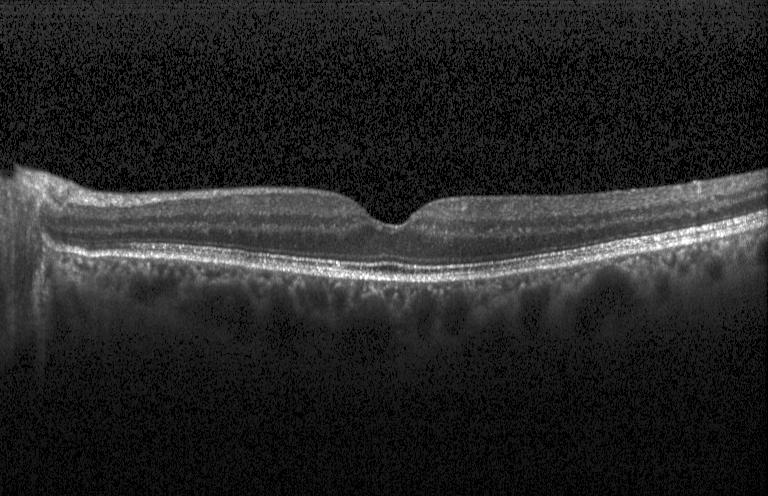 Retinal OCT cross-section showing no choroidal neovascularization, no diabetic macular edema, and no drusen.